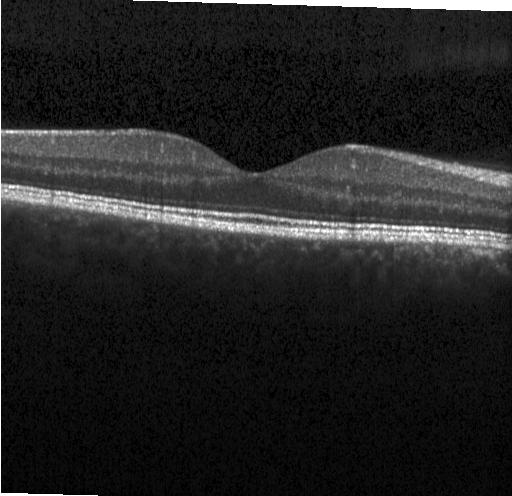
OCT line scan.
Diagnosis: neither CNV, DME, nor drusen.